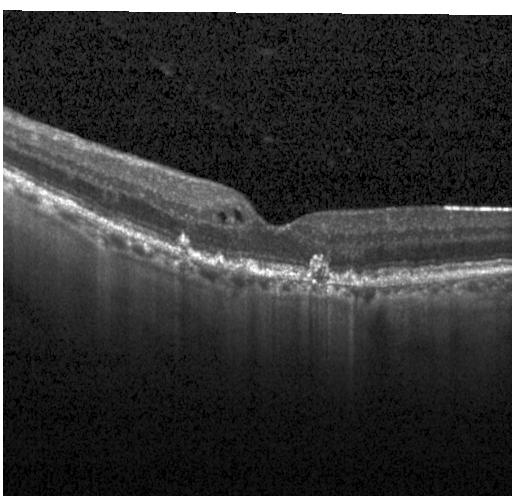 Horizontal scan through the fovea. Optical coherence tomography B-scan. Instrument: Heidelberg Spectralis. SD-OCT.
Diagnosis: choroidal neovascularization (CNV).